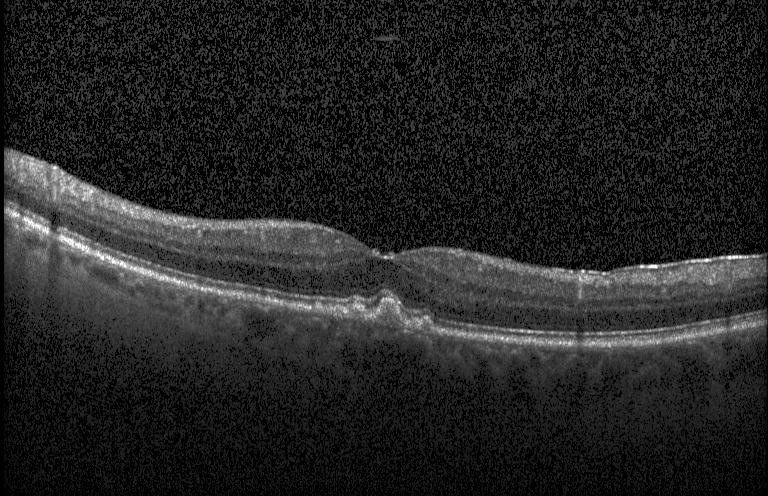 OCT line scan, Heidelberg Spectralis, fovea-centered.
Finding: multiple drusen.